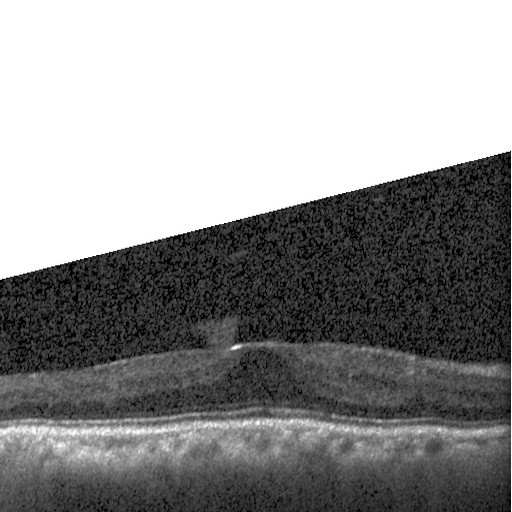

Retinal OCT cross-section
Impression: diabetic macular edema.